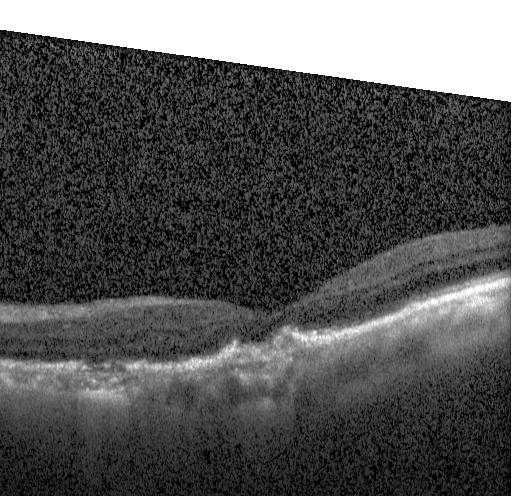 Optical coherence tomography scan. Acquired on a Heidelberg Spectralis. Spectral-domain OCT
Impression: choroidal neovascularization.